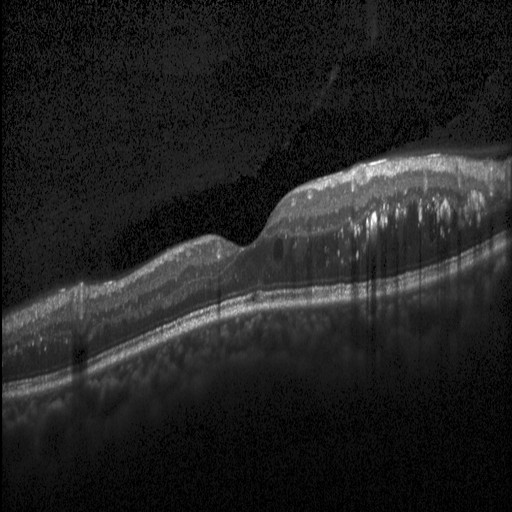 Instrument: Heidelberg Spectralis. Centered on the fovea. OCT B-scan. Spectral-domain OCT
Impression: diabetic macular edema.